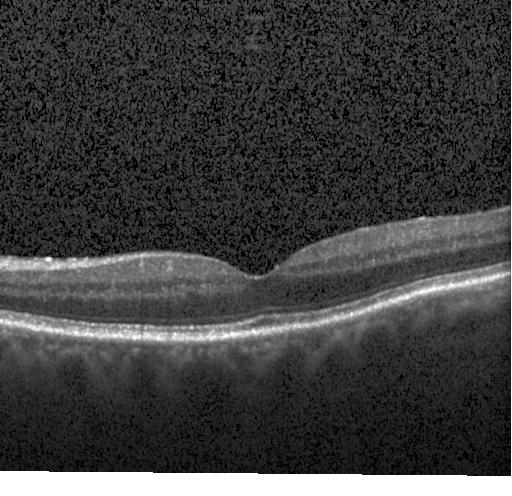 Optical coherence tomography B-scan. Impression: no choroidal neovascularization, diabetic macular edema, or drusen.